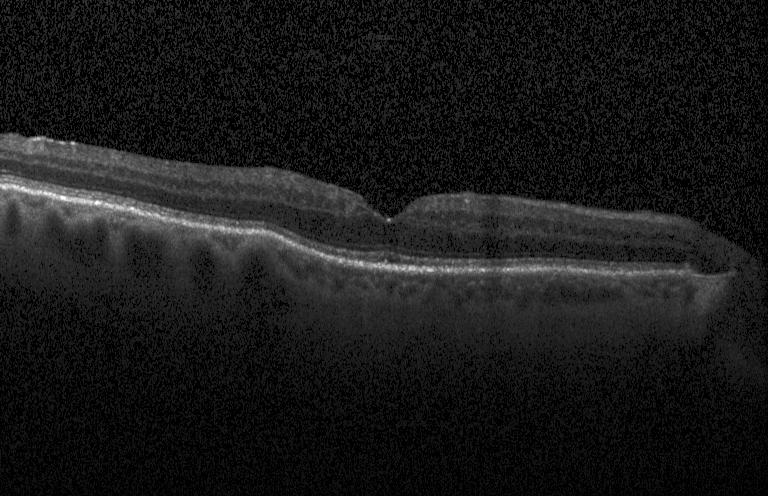

This B-scan demonstrates no evidence of CNV, DME, or drusen.